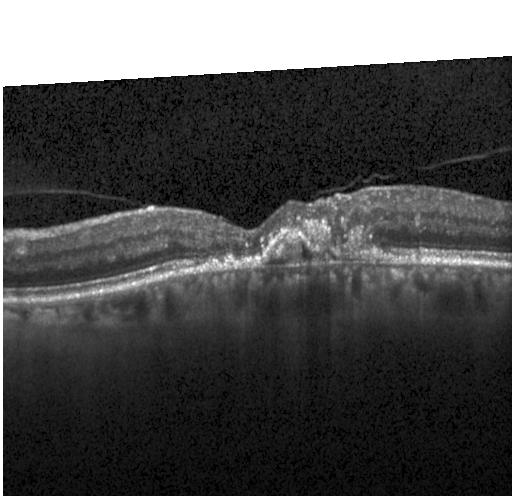

Centered on the fovea. SD-OCT. Acquired on a Heidelberg Spectralis. Retinal OCT B-scan.
This B-scan demonstrates choroidal neovascularization (CNV).